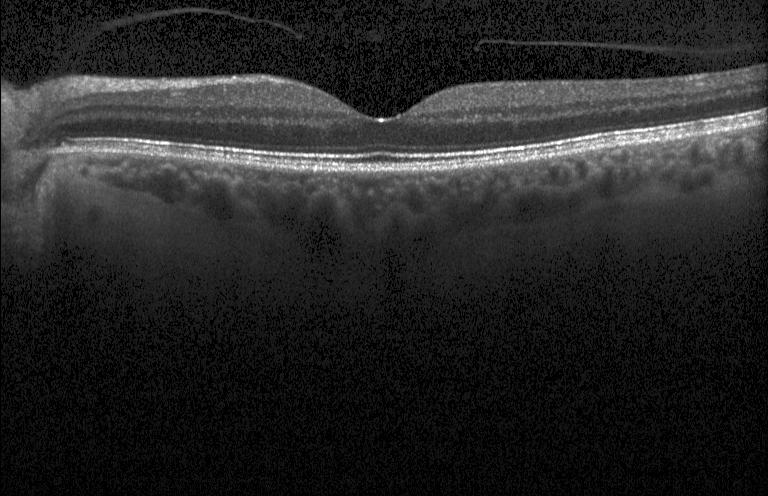
Optical coherence tomography scan, macular scan, instrument: Heidelberg Spectralis.
Finding: no choroidal neovascularization, no diabetic macular edema, and no drusen.